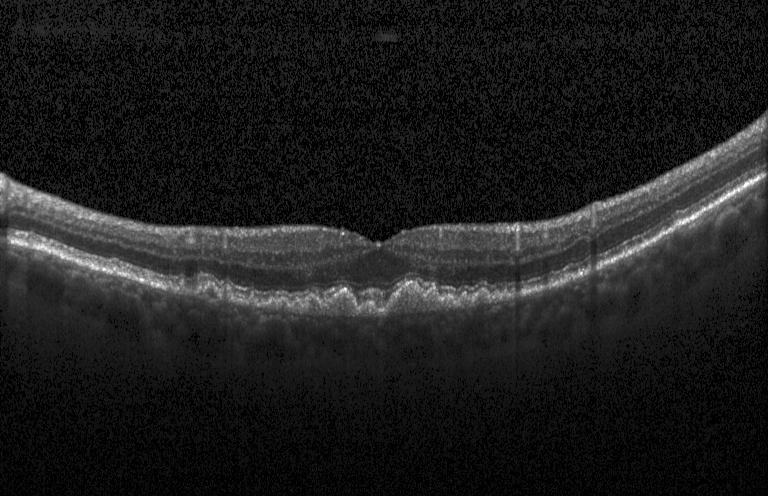
Optical coherence tomography B-scan — Multiple drusen.